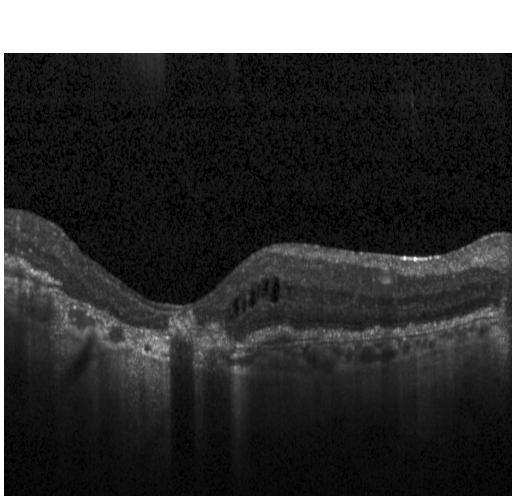 Dx: choroidal neovascularization (CNV).